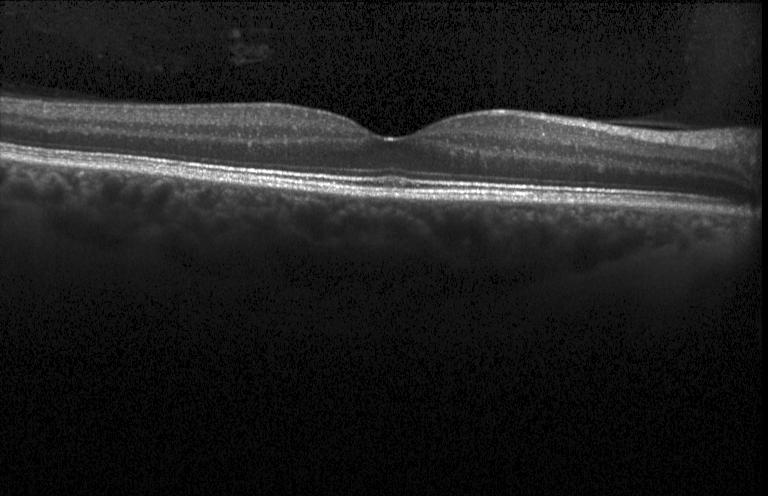 Diagnosis: neither choroidal neovascularization, diabetic macular edema, nor drusen.